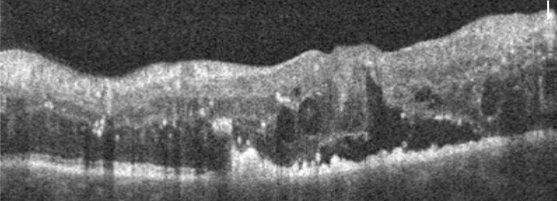
Optical coherence tomography scan. Dx: DME.